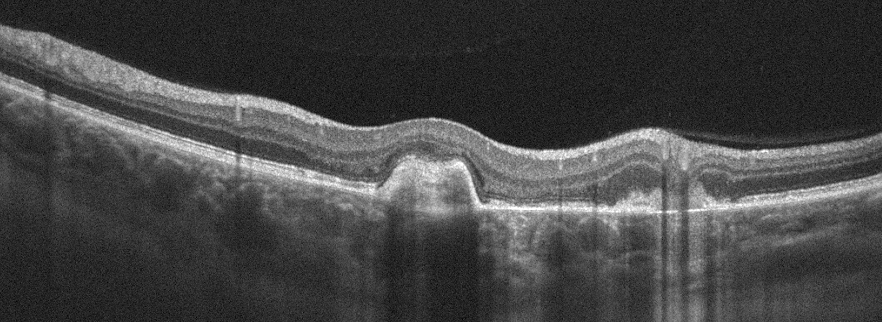
Left eye. Retinal OCT cross-section. The scan shows age-related macular degeneration.